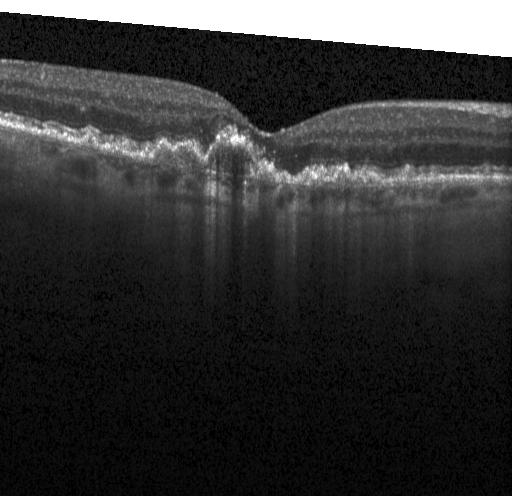 The scan shows CNV.